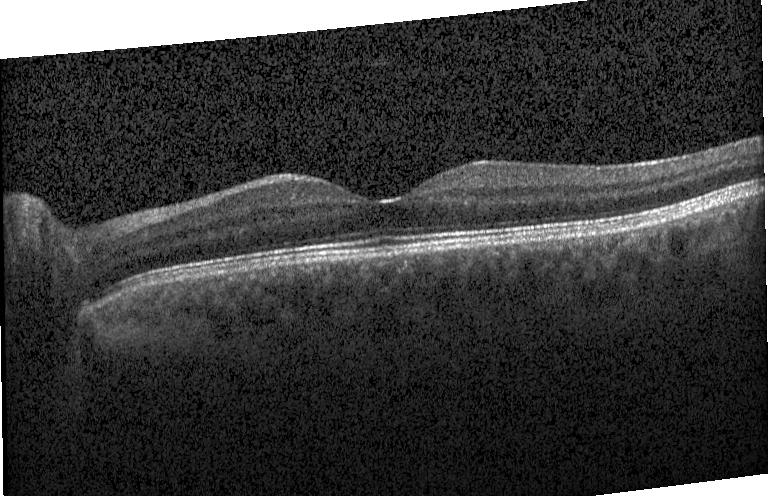
Acquired on a Heidelberg Spectralis, retinal OCT cross-section — Diagnosis: no choroidal neovascularization, diabetic macular edema, or drusen.